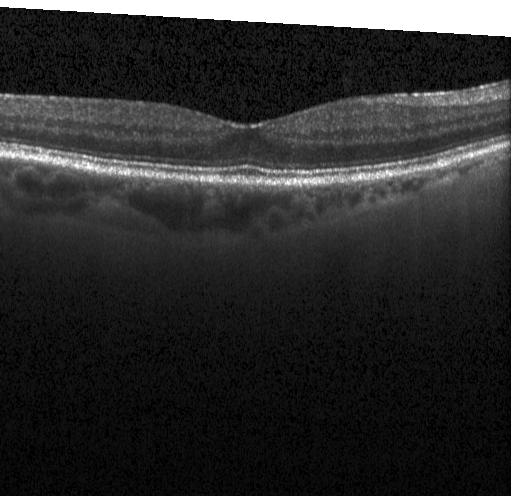
SD-OCT; retinal OCT cross-section. Impression: no evidence of CNV, DME, or drusen.